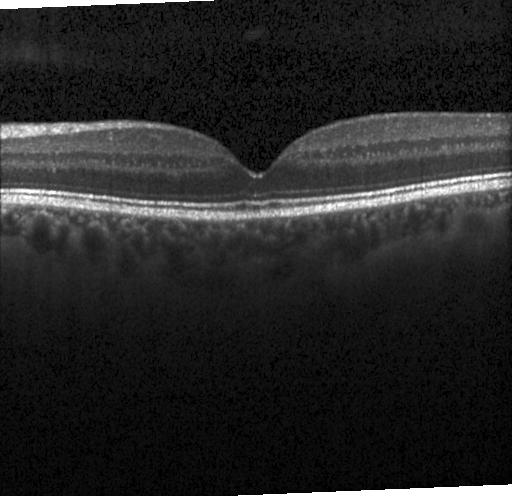
Impression: neither choroidal neovascularization, diabetic macular edema, nor drusen.